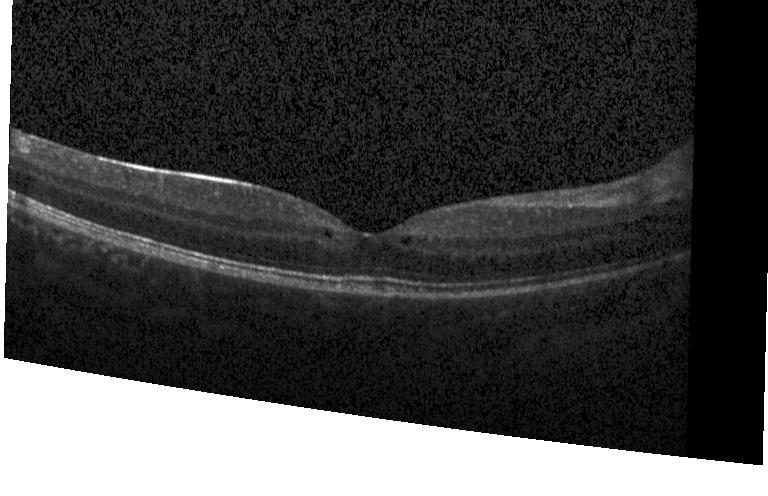
OCT finding: diabetic macular edema.